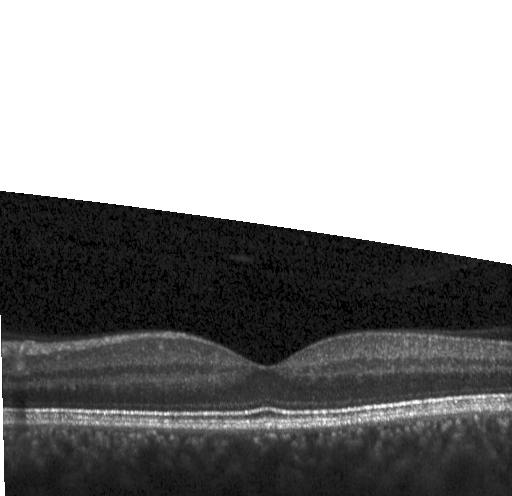

Diagnosis: no CNV, no DME, and no drusen.